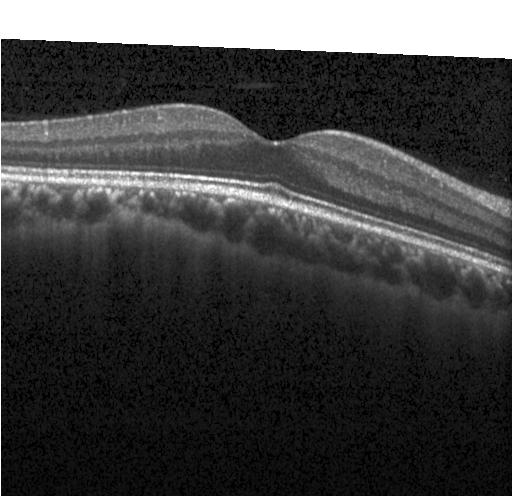

Horizontal scan through the fovea · retinal OCT B-scan · spectral-domain OCT — No evidence of CNV, DME, or drusen.